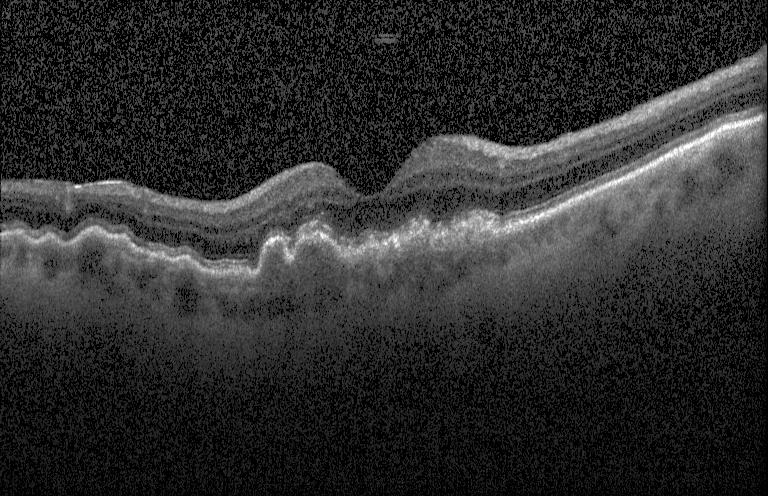

Optical coherence tomography B-scan
This B-scan demonstrates CNV.